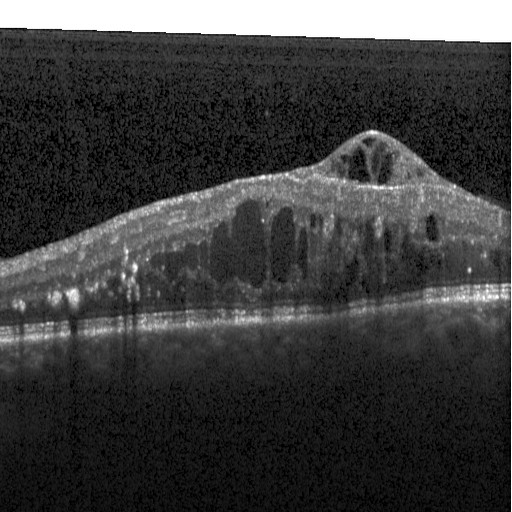
Retinal OCT cross-section.
Diabetic macular edema.